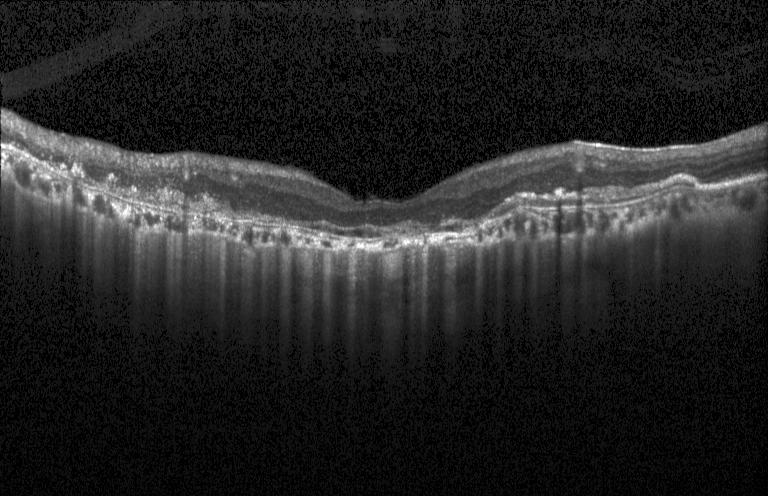

Optical coherence tomography scan. Diagnosis: choroidal neovascularization (CNV).